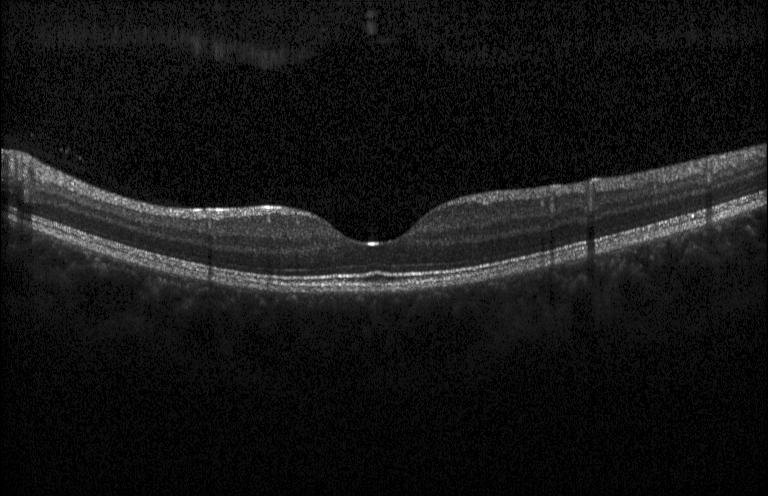

Retinal OCT cross-section showing no choroidal neovascularization, no diabetic macular edema, and no drusen.